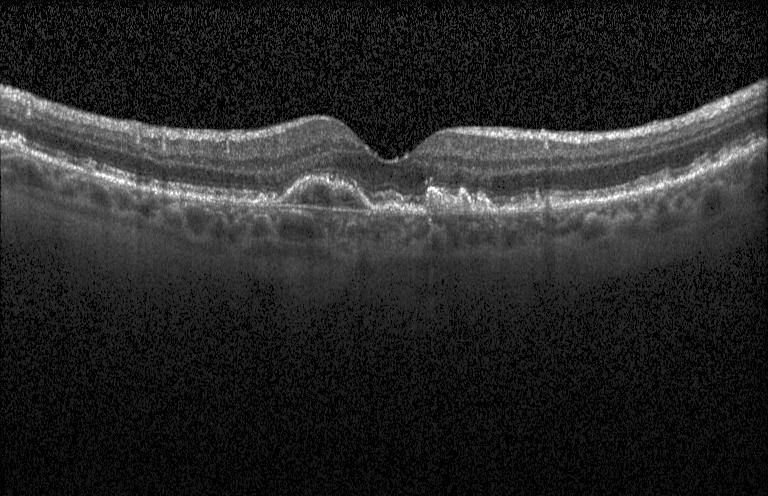
OCT line scan
Diagnosis: choroidal neovascularization.